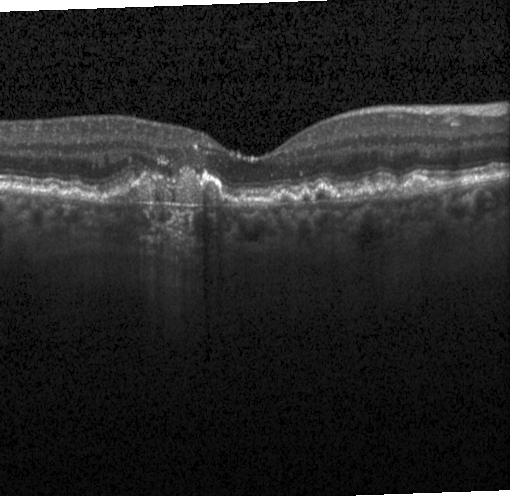

Macular scan · OCT B-scan.
Impression: a choroidal neovascular membrane.